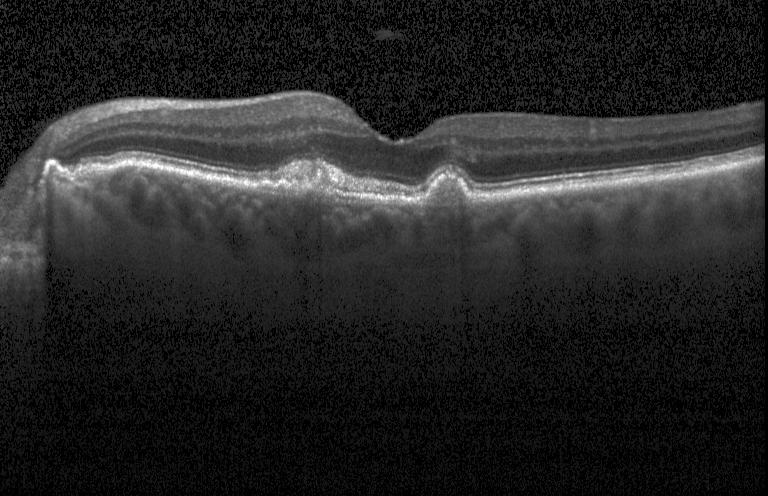

SD-OCT · retinal OCT B-scan · Heidelberg Spectralis OCT system — Finding: choroidal neovascularization (CNV).